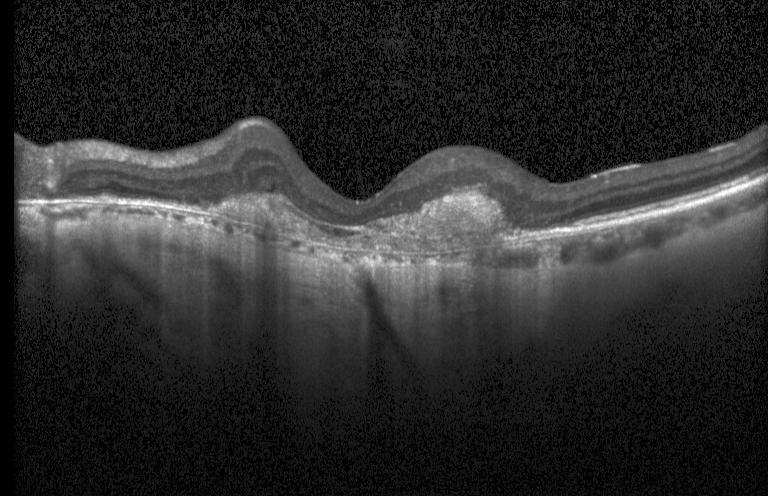
This B-scan demonstrates choroidal neovascularization (CNV).